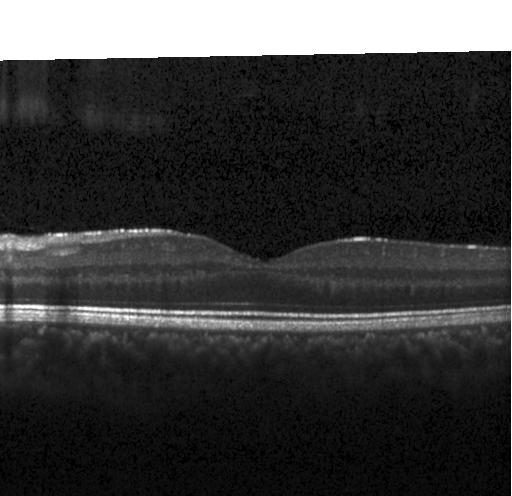
Finding: no evidence of CNV, DME, or drusen.